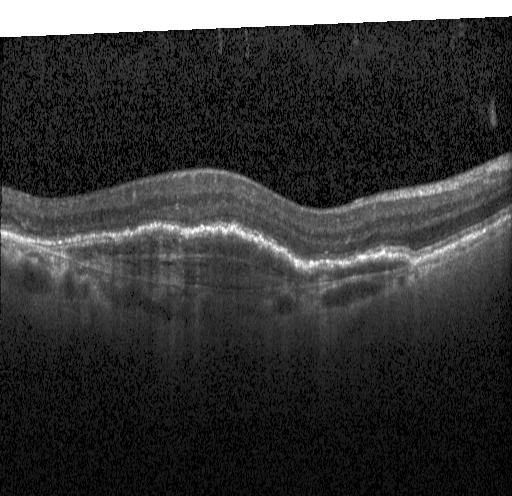
Macular scan · OCT B-scan
Impression: a choroidal neovascular membrane.